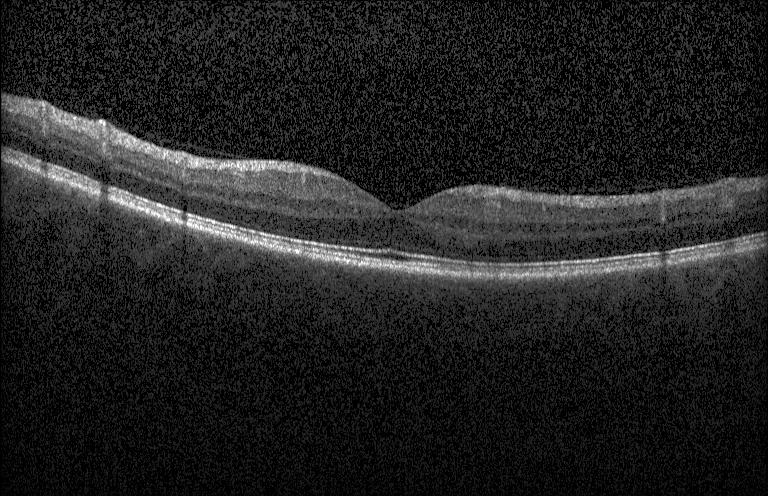

OCT line scan · horizontal scan through the fovea · spectral-domain OCT · Heidelberg Spectralis — Assessment: neither CNV, DME, nor drusen.